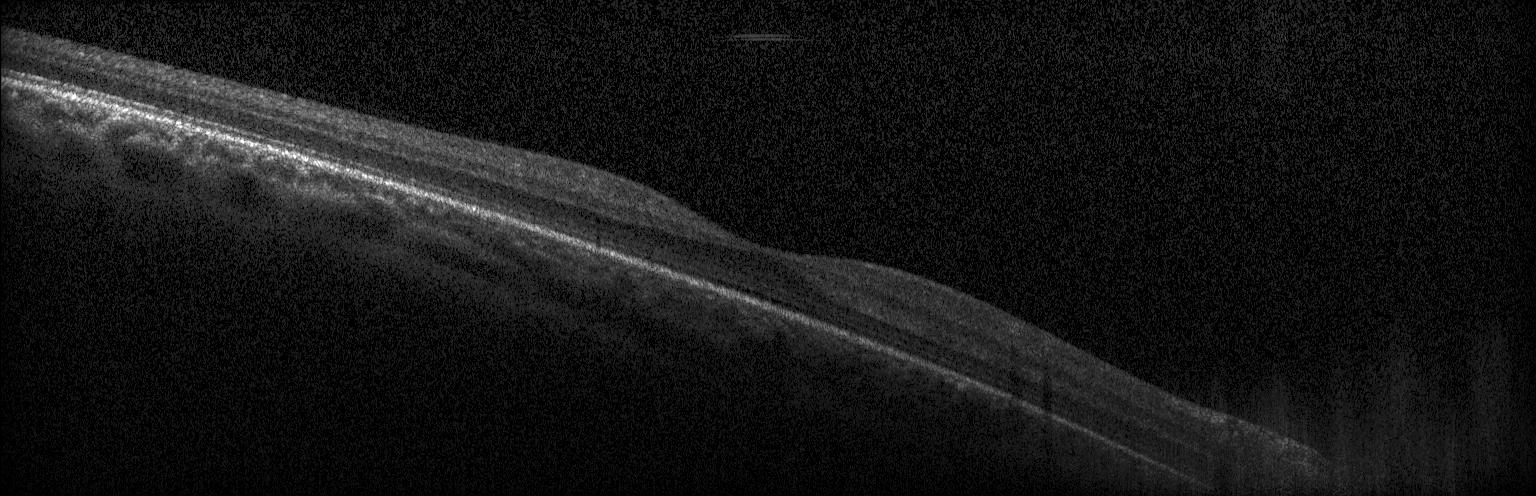 SD-OCT, retinal OCT B-scan, through the macula
The scan shows no choroidal neovascularization, no diabetic macular edema, and no drusen.